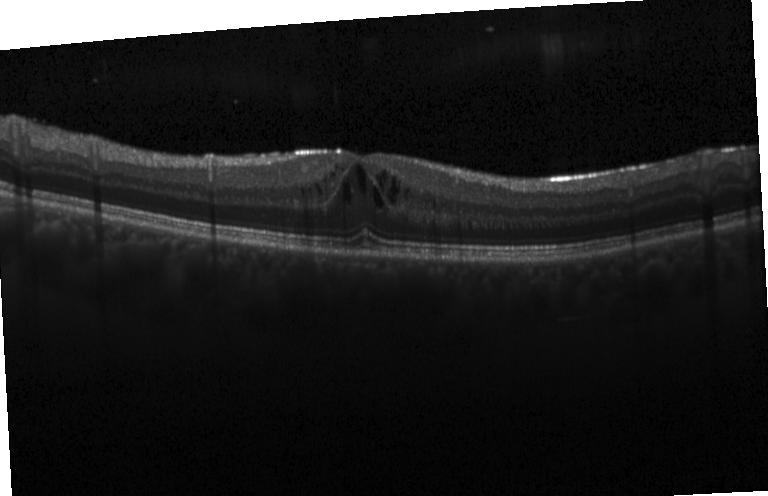
OCT B-scan, Heidelberg Spectralis, spectral-domain OCT, macular scan
Impression: diabetic macular edema (DME).